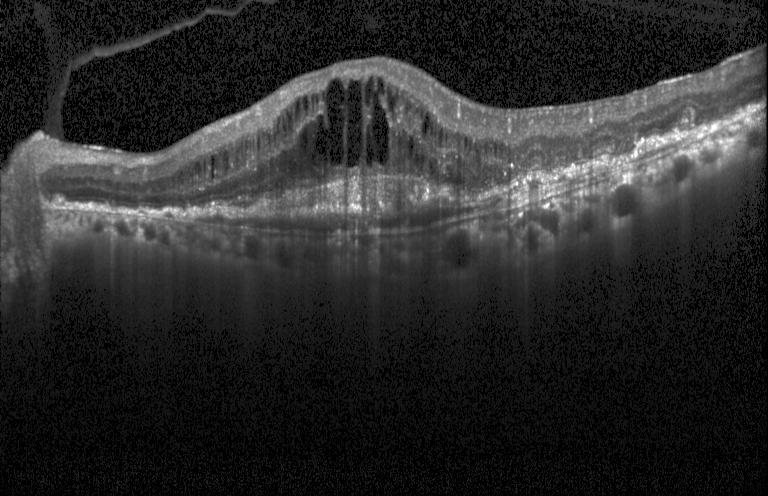

Impression: a choroidal neovascular membrane.